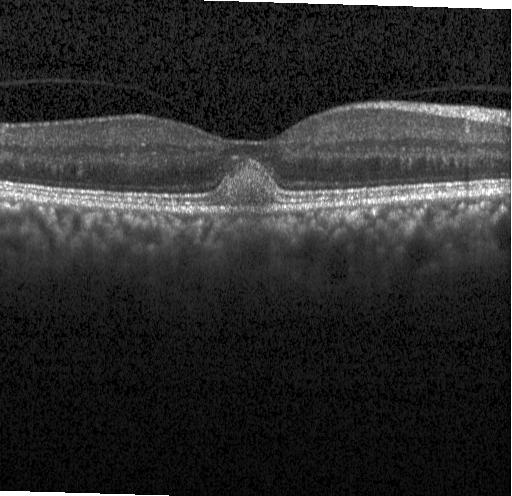 Heidelberg Spectralis · retinal OCT B-scan · SD-OCT · fovea-centered.
A choroidal neovascular membrane.